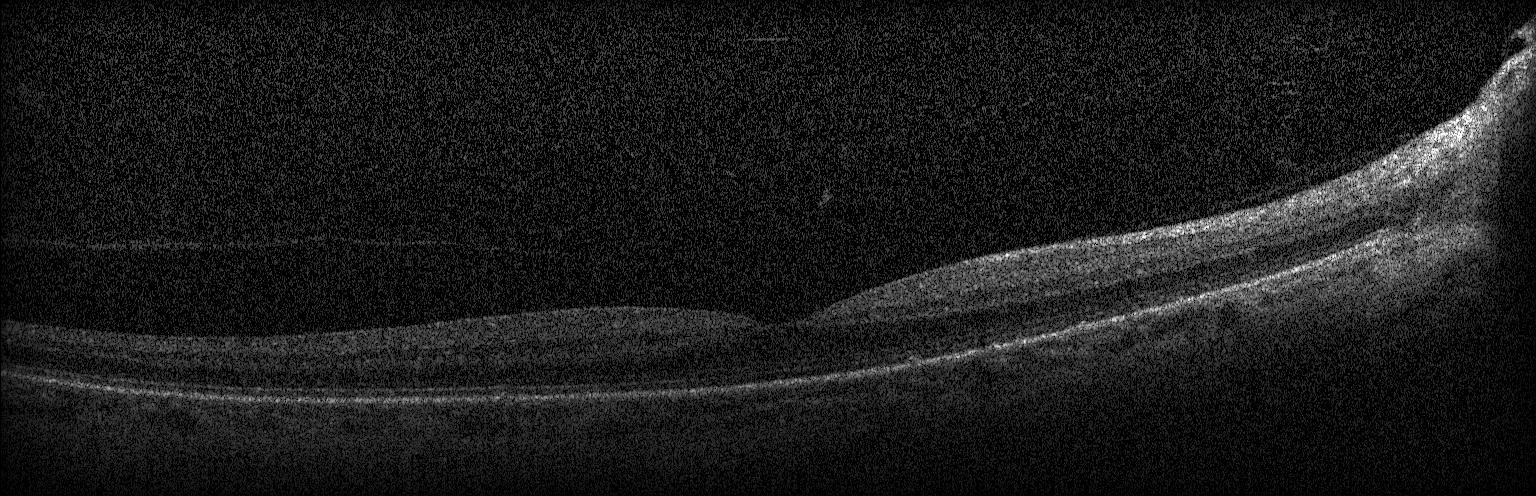 Retinal OCT B-scan.
Diagnosis: no choroidal neovascularization, diabetic macular edema, or drusen.